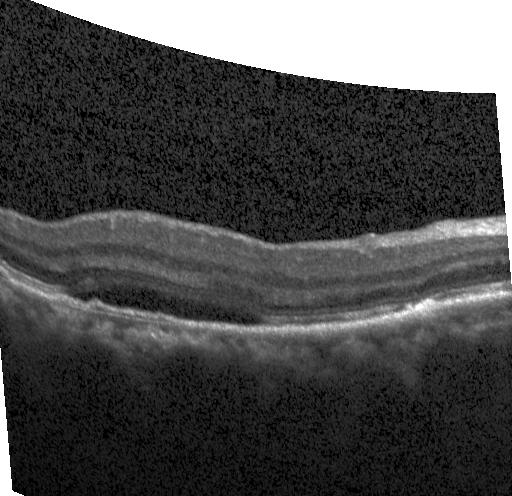

Centered on the fovea · SD-OCT · OCT line scan.
Finding: choroidal neovascularization (CNV).